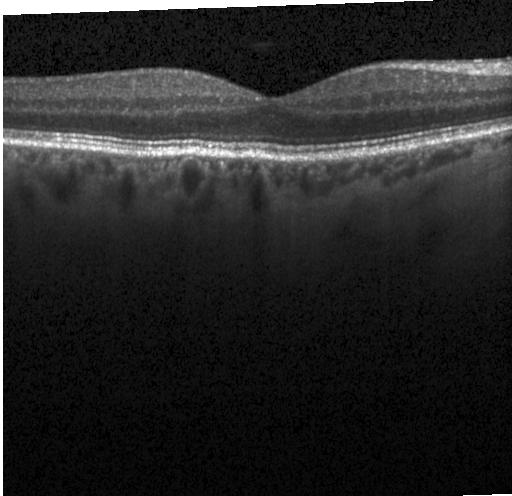 Spectral-domain OCT B-scan: neither choroidal neovascularization, diabetic macular edema, nor drusen.